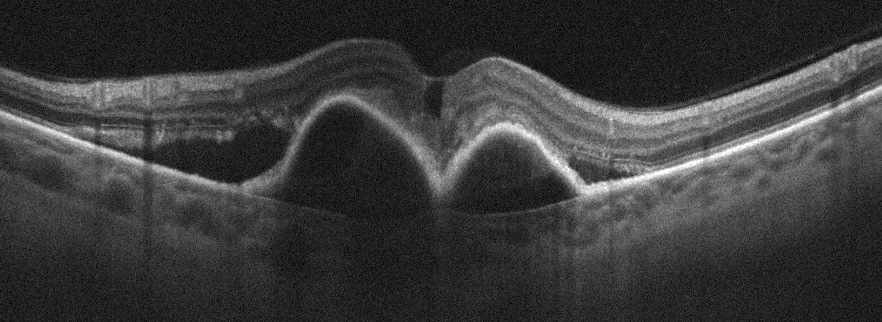
Optical coherence tomography scan. Finding: age-related macular degeneration (AMD).